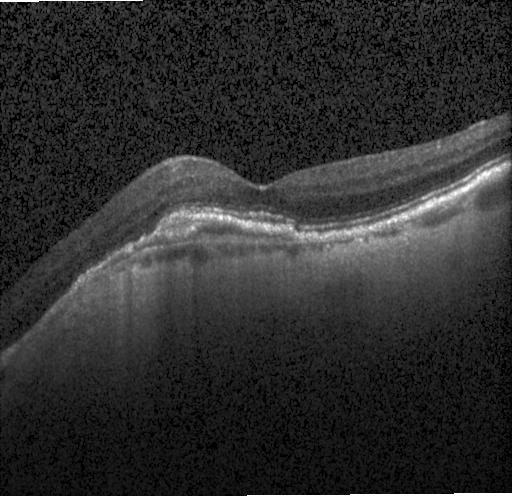
Retinal OCT cross-section showing choroidal neovascularization.